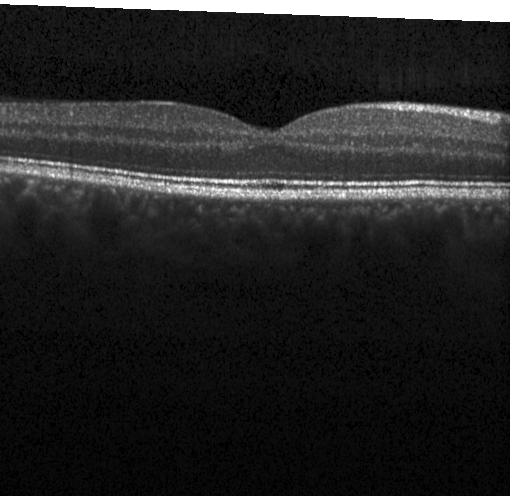 Impression: neither choroidal neovascularization, diabetic macular edema, nor drusen.